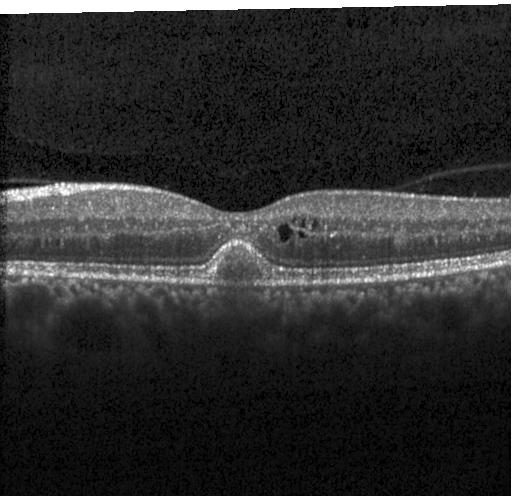 Assessment: choroidal neovascularization.